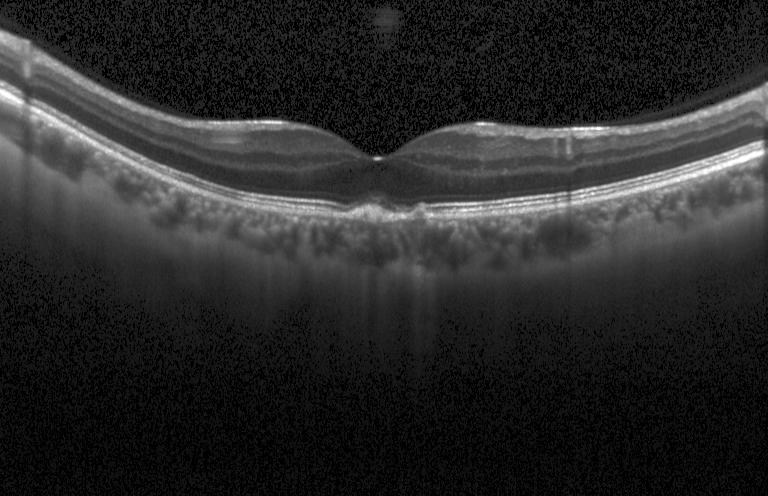

OCT line scan
Impression: CNV.